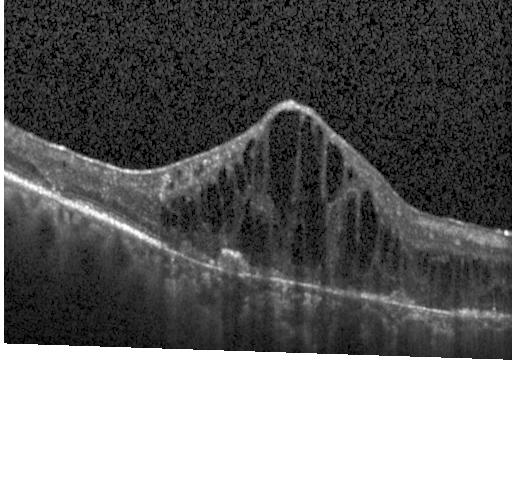 OCT B-scan showing choroidal neovascularization (CNV).